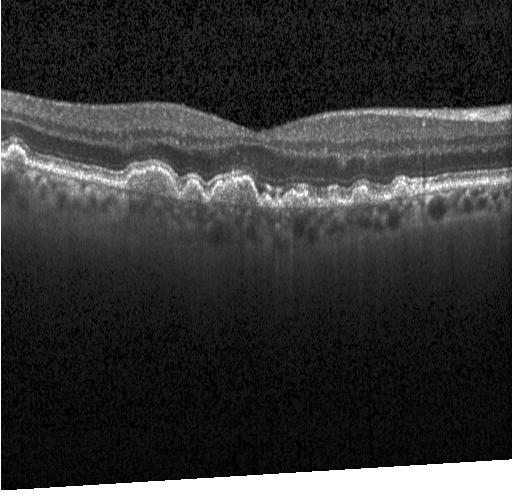 Impression: multiple drusen.